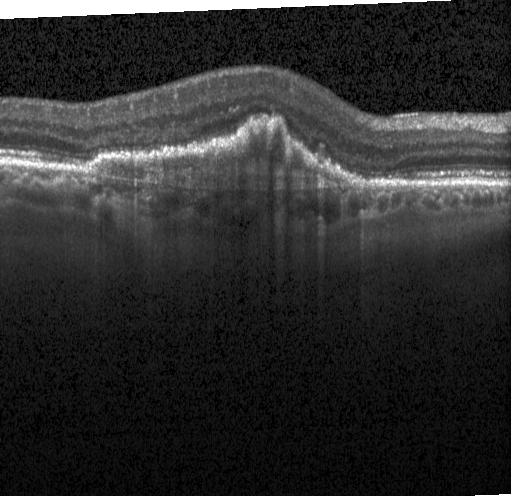
OCT line scan
Finding: a choroidal neovascular membrane.